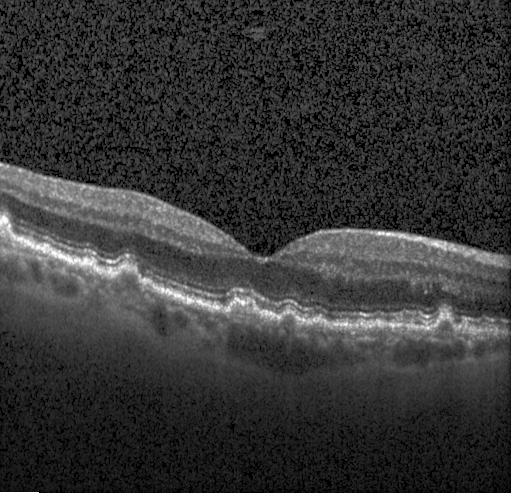 Optical coherence tomography scan; macular scan.
Dx: sub-RPE drusenoid deposits.